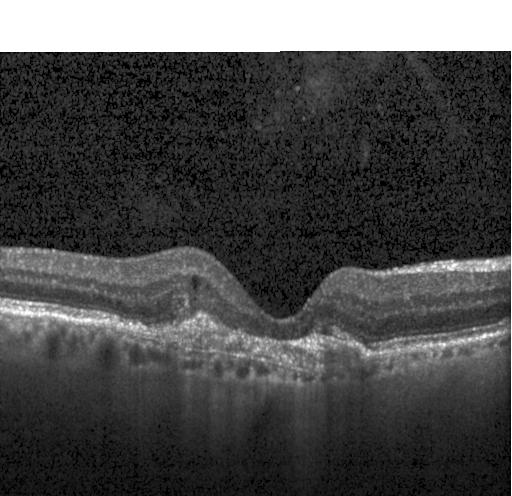
Spectral-domain OCT B-scan: choroidal neovascularization (CNV).